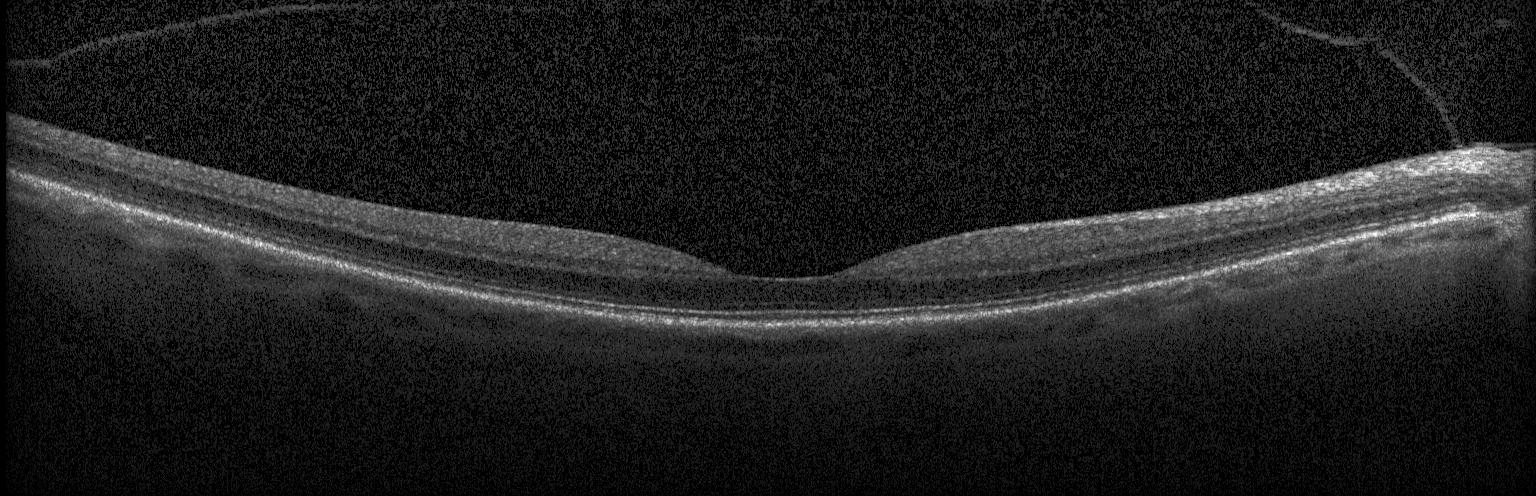 Macular OCT demonstrating no evidence of choroidal neovascularization, diabetic macular edema, or drusen.